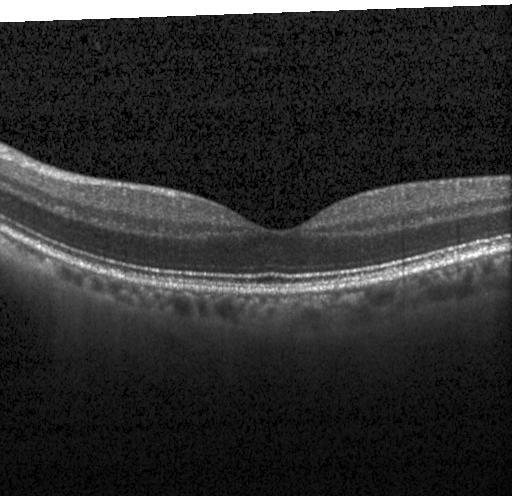
Instrument: Heidelberg Spectralis. Optical coherence tomography B-scan — Assessment: no evidence of choroidal neovascularization, diabetic macular edema, or drusen.